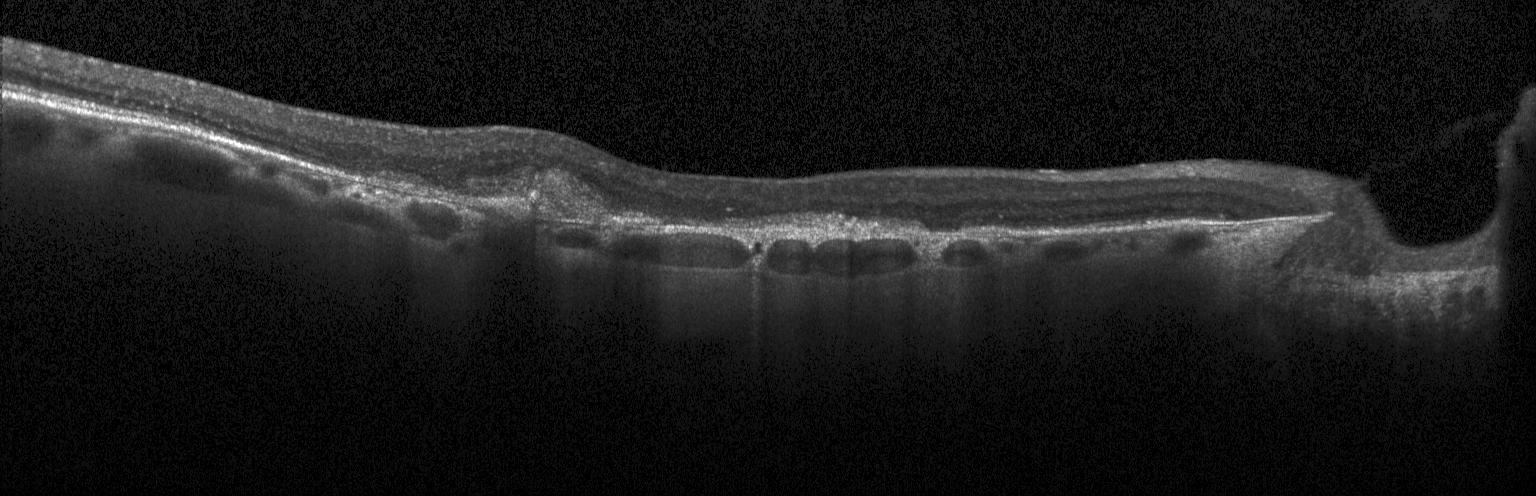

Heidelberg Spectralis OCT system; horizontal scan through the fovea; SD-OCT; OCT B-scan.
Choroidal neovascularization (CNV).